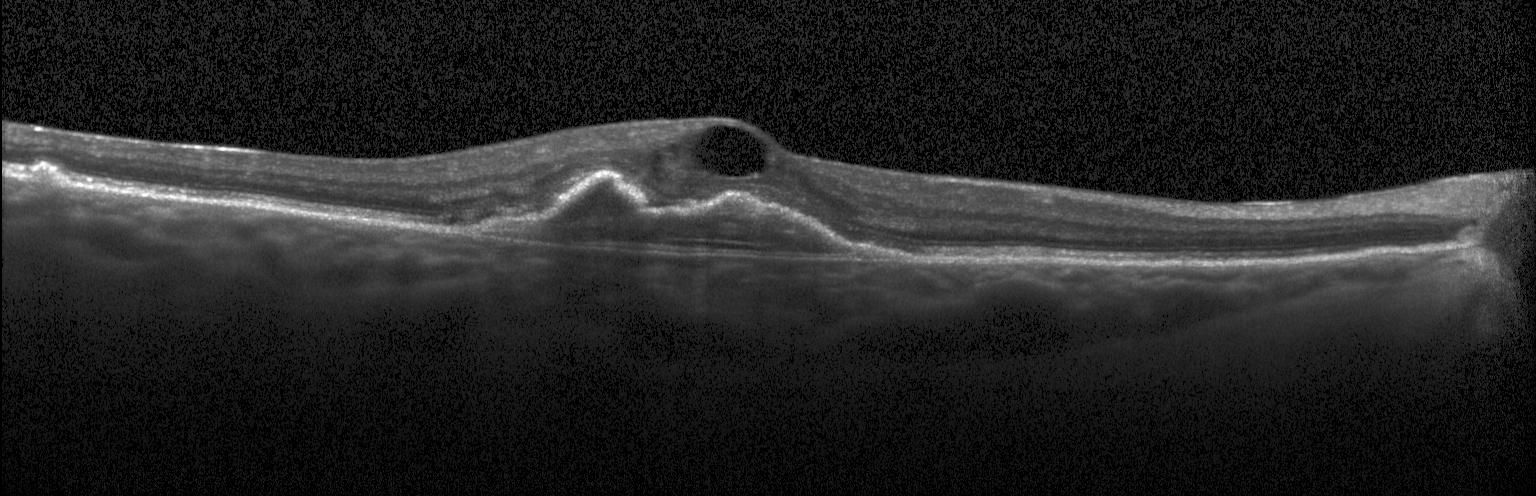 Retinal OCT B-scan.
This B-scan demonstrates a choroidal neovascular membrane.